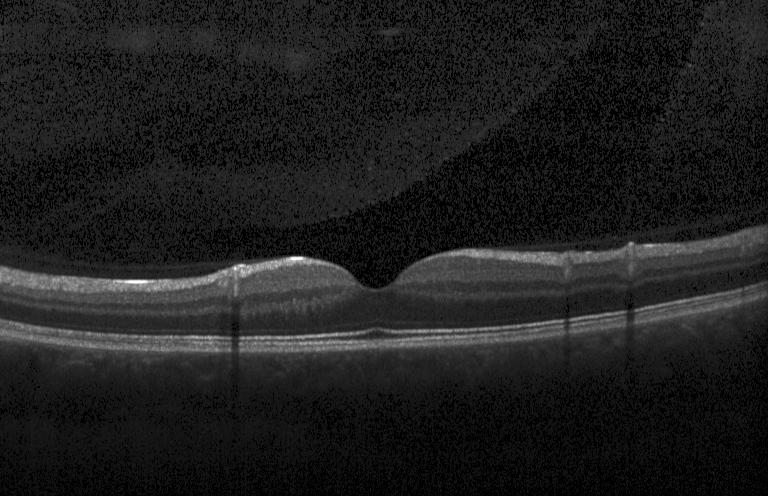

Dx: no CNV, no DME, and no drusen.